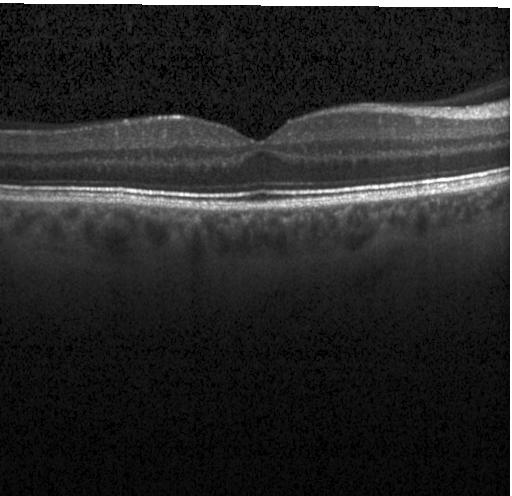

Retinal OCT B-scan · spectral-domain OCT · Heidelberg Spectralis OCT system. Impression: neither choroidal neovascularization, diabetic macular edema, nor drusen.